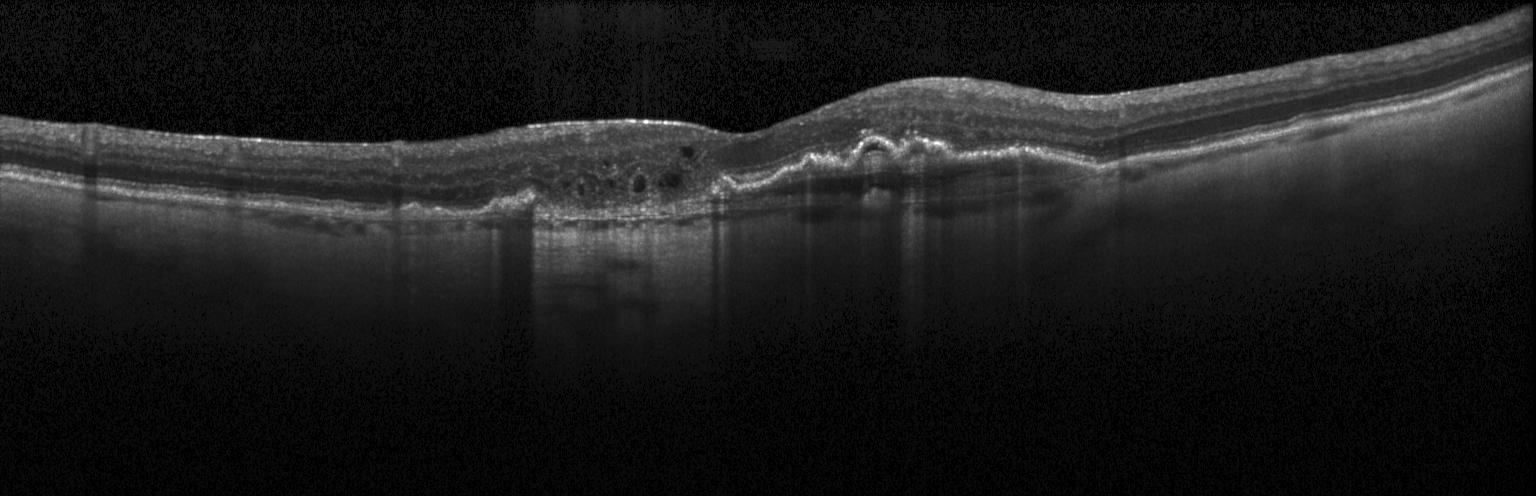 Spectral-domain OCT · optical coherence tomography scan
Diagnosis: choroidal neovascularization.